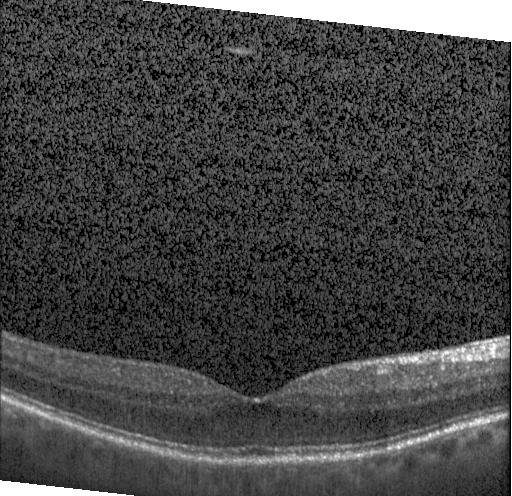

Assessment: neither choroidal neovascularization, diabetic macular edema, nor drusen.